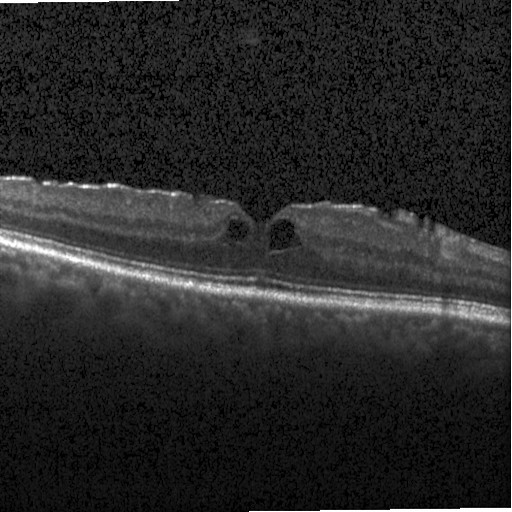

Finding: diabetic macular edema.